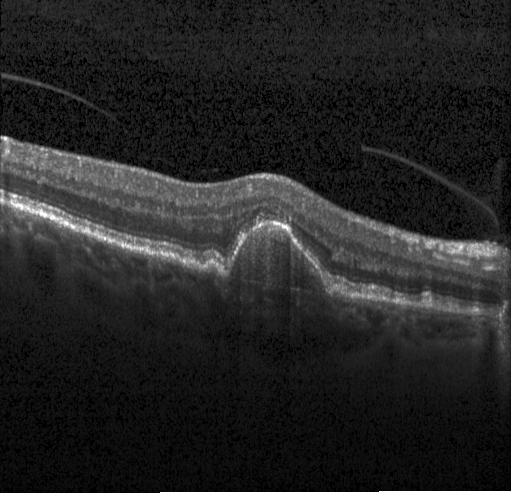 OCT scan showing choroidal neovascularization.